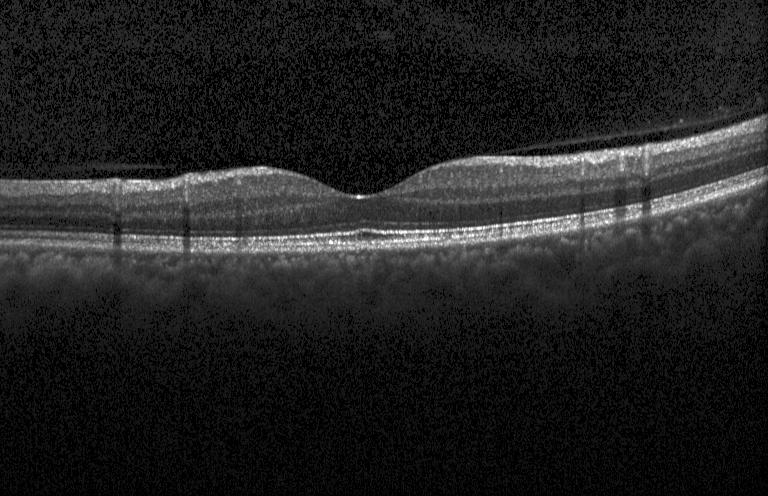 Diagnosis: no choroidal neovascularization, diabetic macular edema, or drusen.